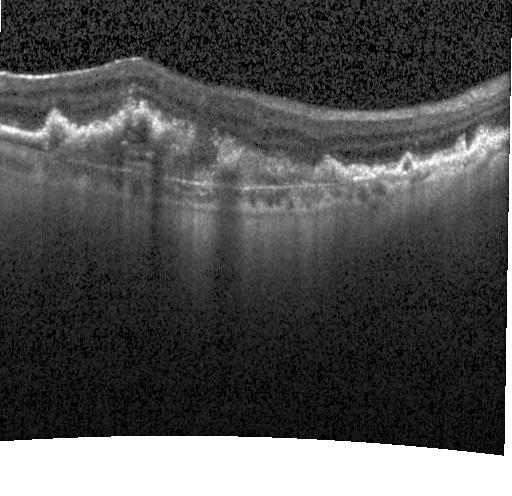

Macular OCT demonstrating a choroidal neovascular membrane.